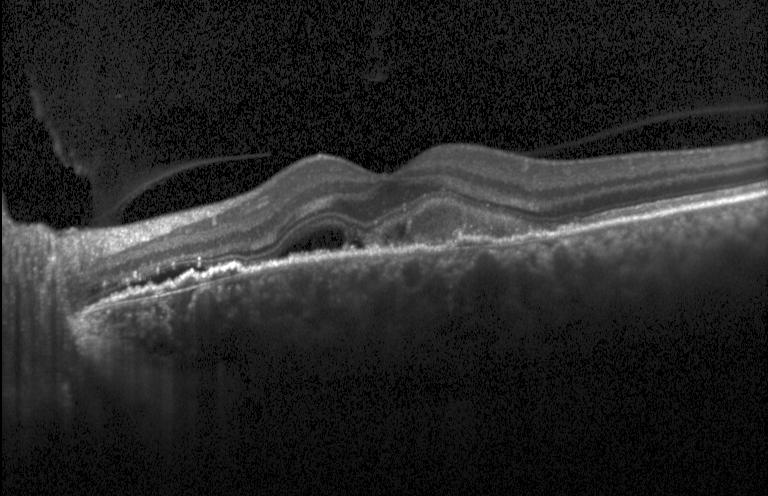

Macular OCT demonstrating choroidal neovascularization.